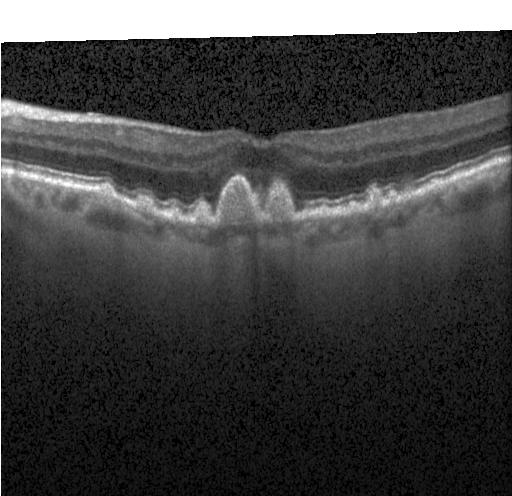 Horizontal scan through the fovea · retinal OCT B-scan · instrument: Heidelberg Spectralis · SD-OCT.
Impression: sub-RPE drusenoid deposits.